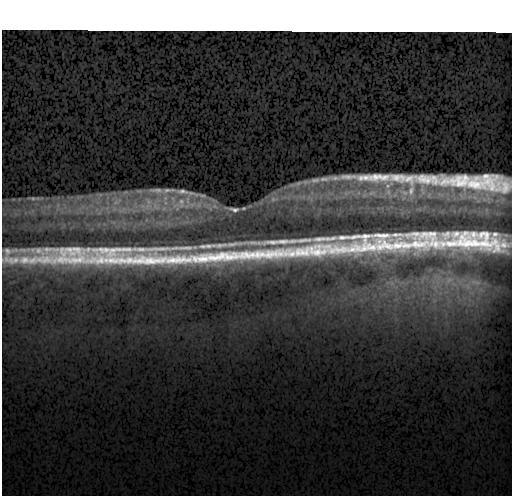 OCT B-scan. This B-scan demonstrates neither CNV, DME, nor drusen.